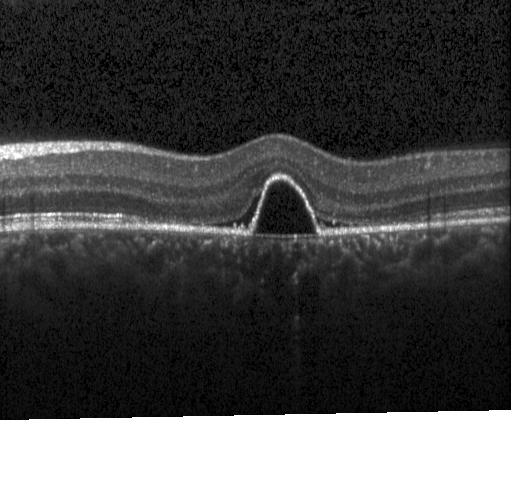
Macular OCT: a choroidal neovascular membrane.